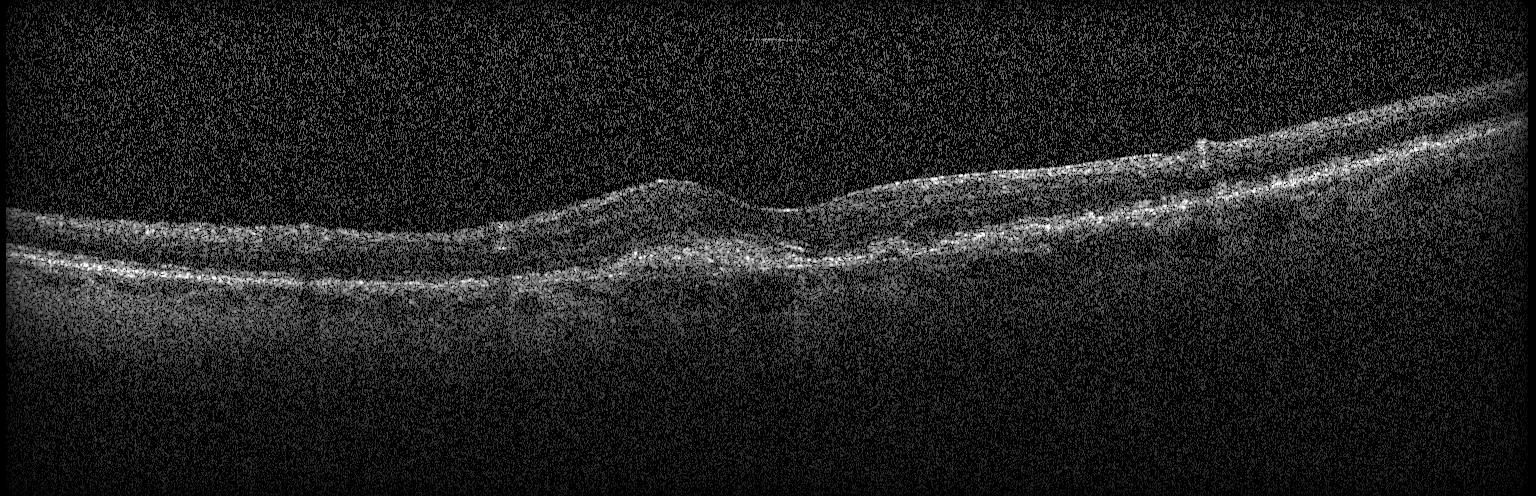

Optical coherence tomography scan. The scan shows a choroidal neovascular membrane.